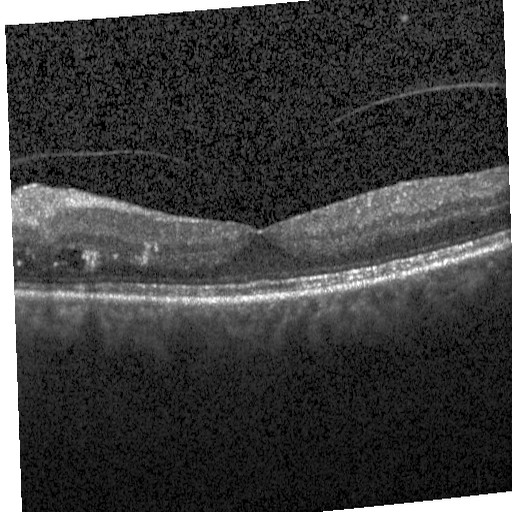
Retinal OCT cross-section
Macular OCT: diabetic macular edema.